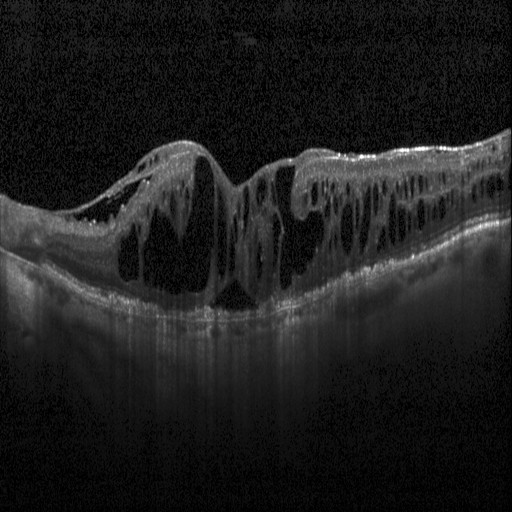 Instrument: Heidelberg Spectralis. Optical coherence tomography B-scan. Finding: DME.